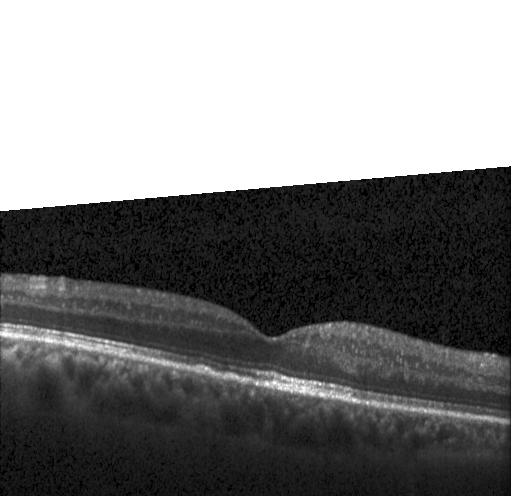

Macular OCT: no evidence of CNV, DME, or drusen.